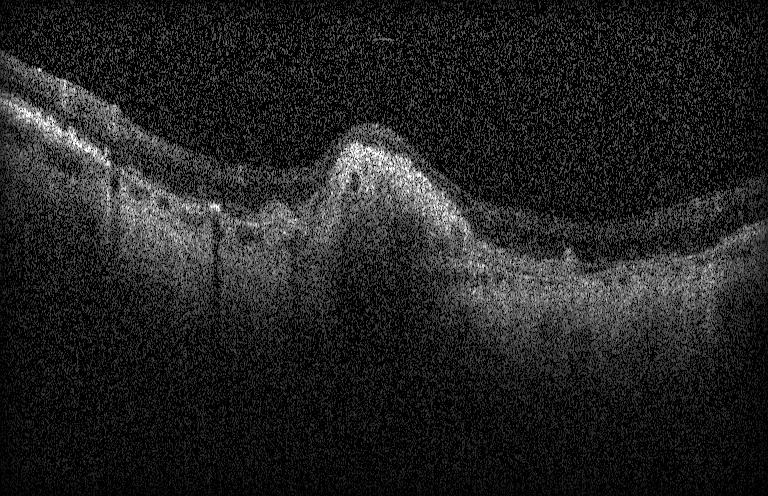
Spectral-domain optical coherence tomography. Horizontal scan through the fovea. Instrument: Heidelberg Spectralis. Optical coherence tomography scan
Diagnosis: CNV.